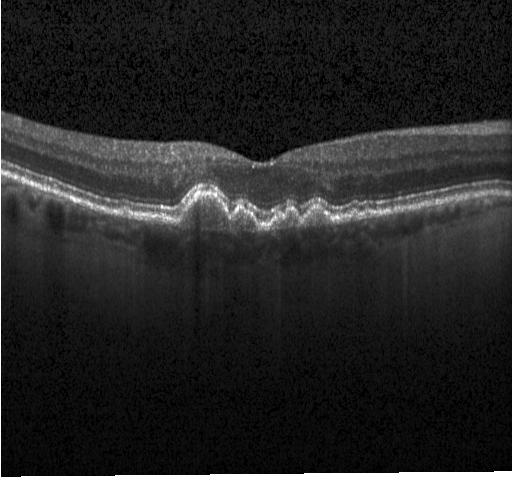

Diagnosis: sub-RPE drusenoid deposits.